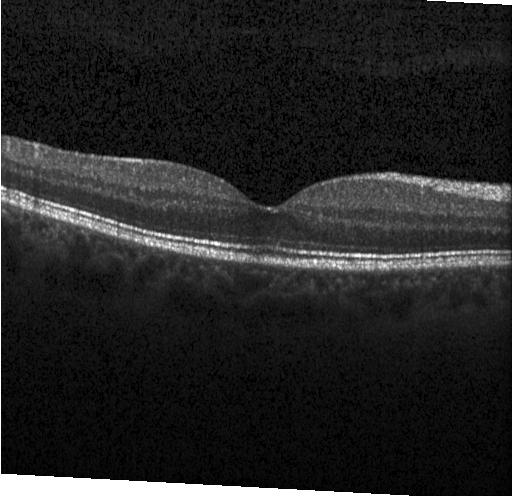

OCT B-scan · acquired on a Heidelberg Spectralis
This B-scan demonstrates neither choroidal neovascularization, diabetic macular edema, nor drusen.